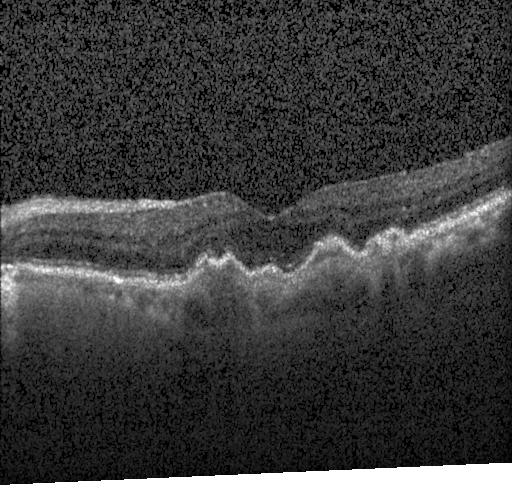

OCT line scan; acquired on a Heidelberg Spectralis — Macular OCT: choroidal neovascularization.